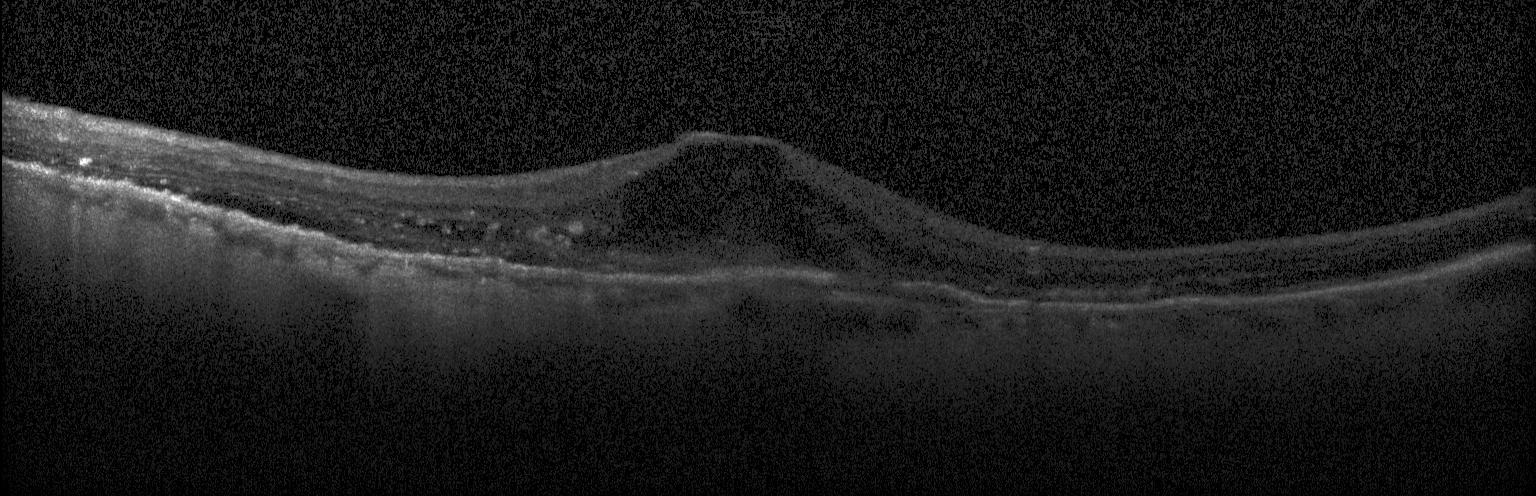

Optical coherence tomography B-scan.
Diagnosis: CNV.